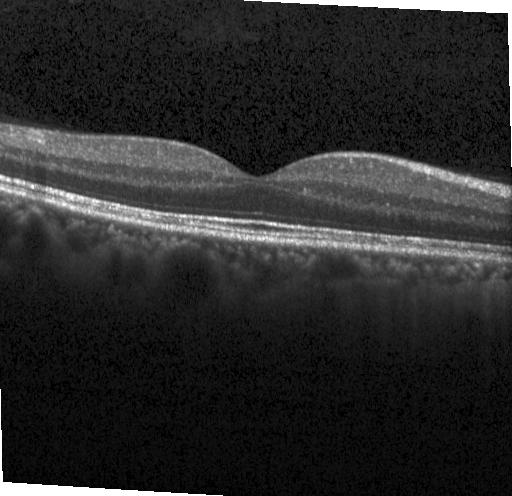 Fovea-centered; retinal OCT B-scan. OCT finding: no evidence of CNV, DME, or drusen.